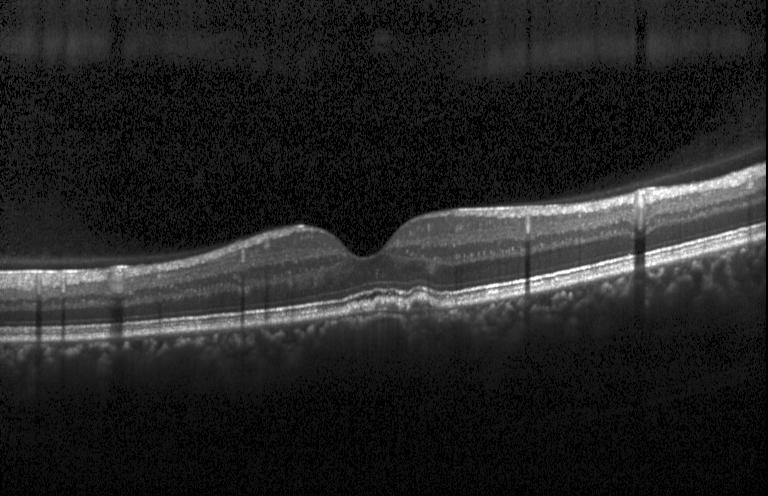

Dx: multiple drusen.